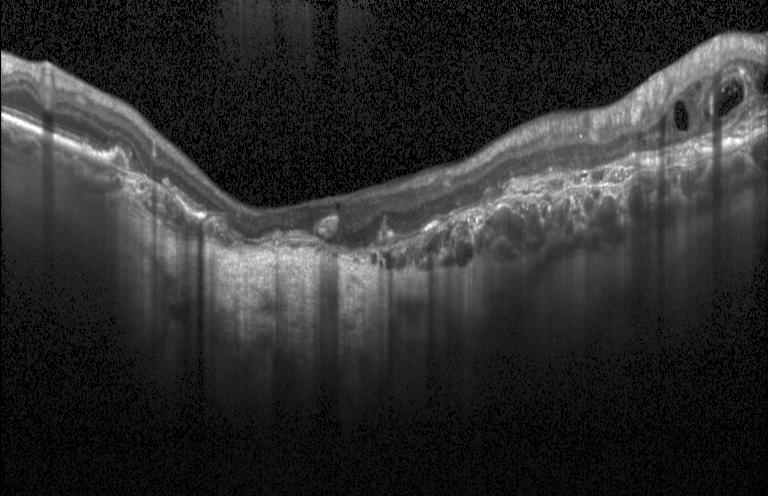 Spectral-domain OCT B-scan: choroidal neovascularization (CNV).